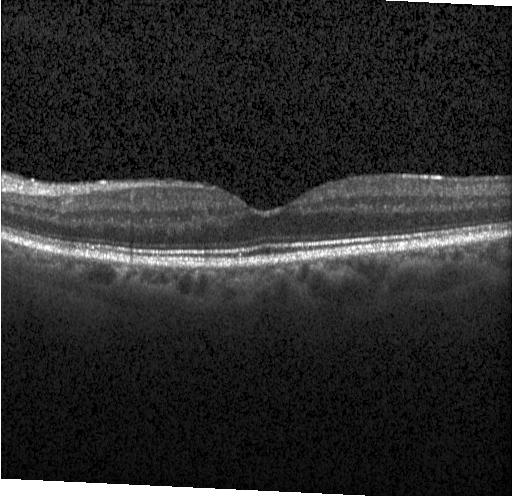 Fovea-centered, retinal OCT B-scan, spectral-domain OCT, Heidelberg Spectralis OCT system.
The scan shows neither CNV, DME, nor drusen.